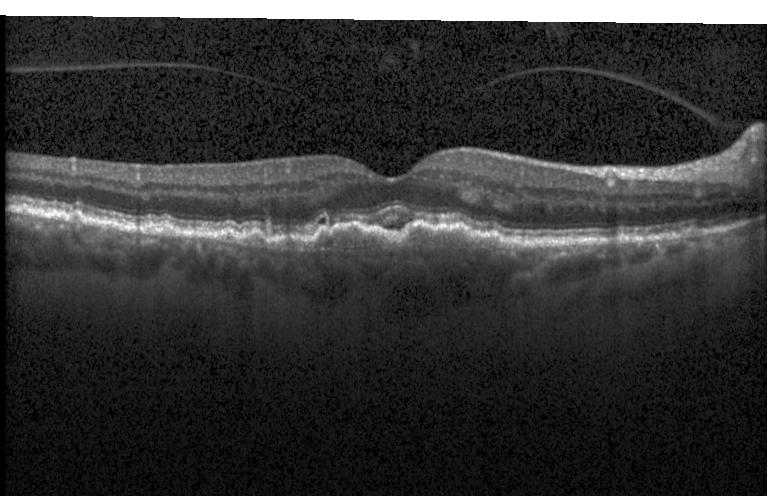 Diagnosis: a choroidal neovascular membrane.